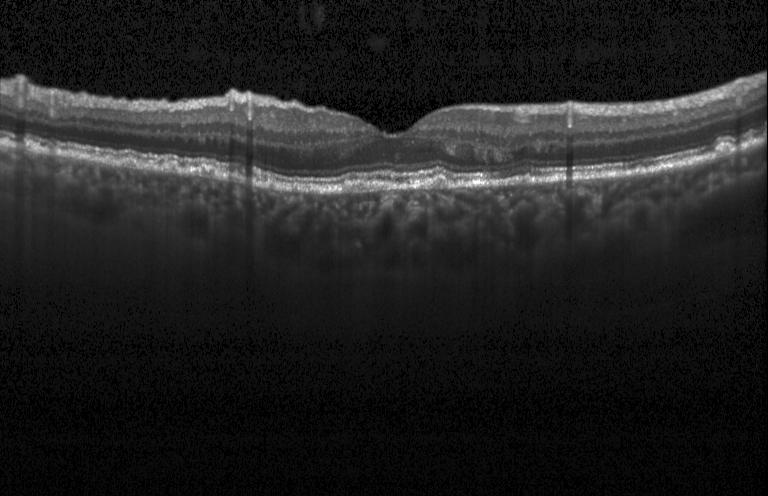
Finding: multiple drusen.